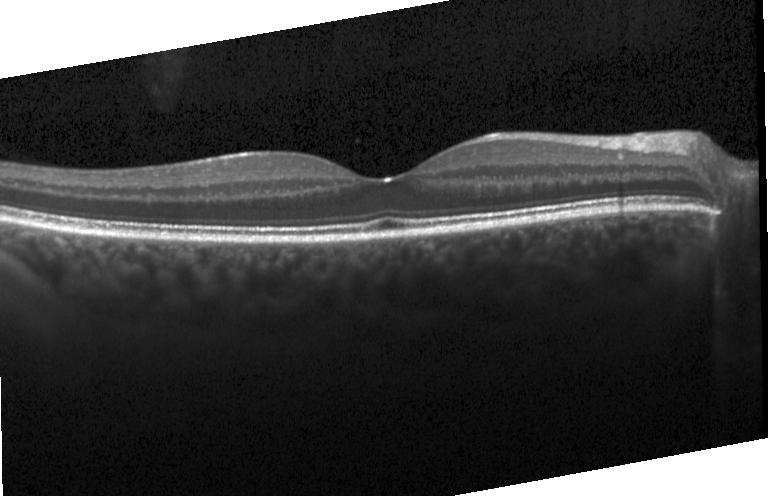
Macular OCT demonstrating no evidence of choroidal neovascularization, diabetic macular edema, or drusen.